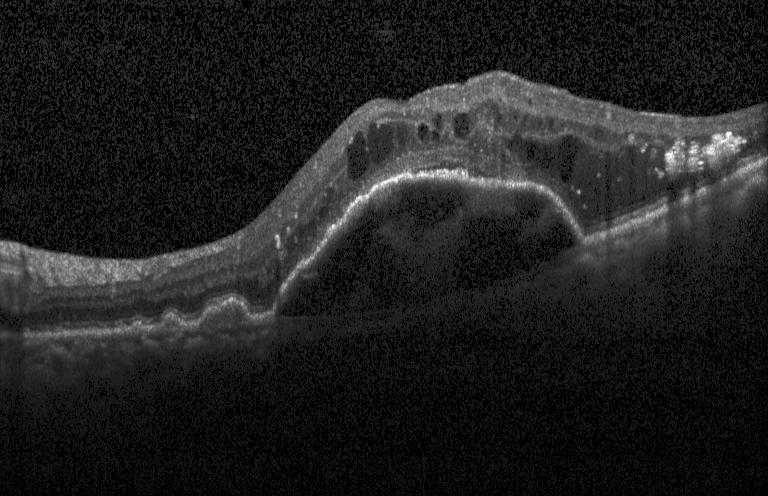
Retinal OCT cross-section
Diagnosis: choroidal neovascularization.